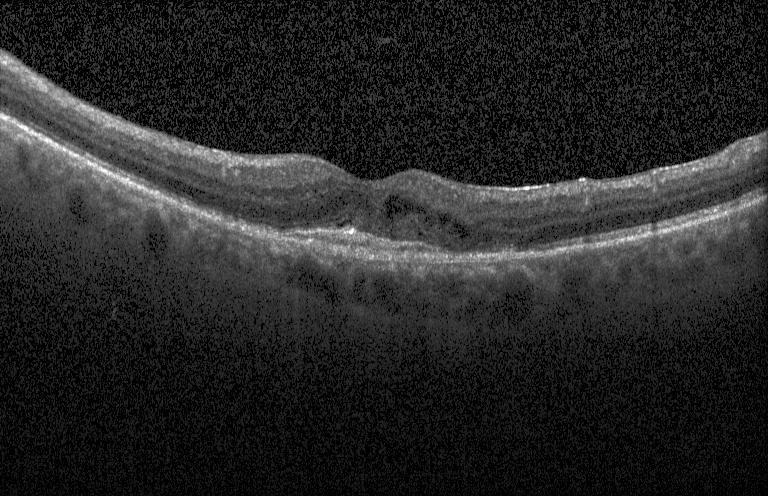
Optical coherence tomography B-scan · centered on the fovea · spectral-domain optical coherence tomography — Dx: a choroidal neovascular membrane.